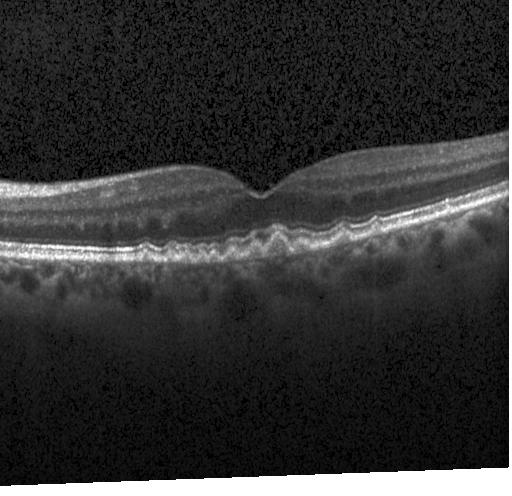
Macular scan. OCT line scan. Spectral-domain OCT.
Assessment: sub-RPE drusenoid deposits.